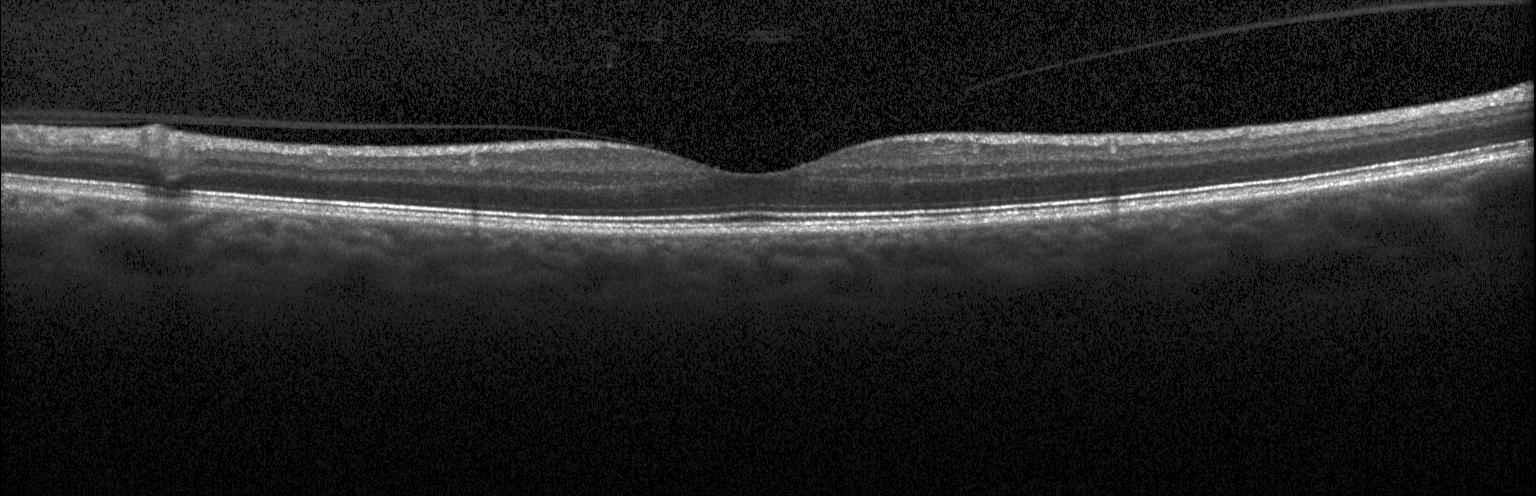 Optical coherence tomography B-scan, acquired on a Heidelberg Spectralis, centered on the fovea
Impression: neither choroidal neovascularization, diabetic macular edema, nor drusen.